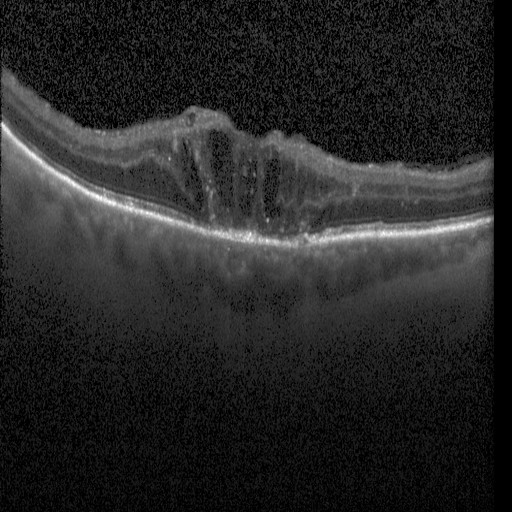
Spectral-domain OCT; optical coherence tomography B-scan; instrument: Heidelberg Spectralis. Impression: diabetic macular edema.